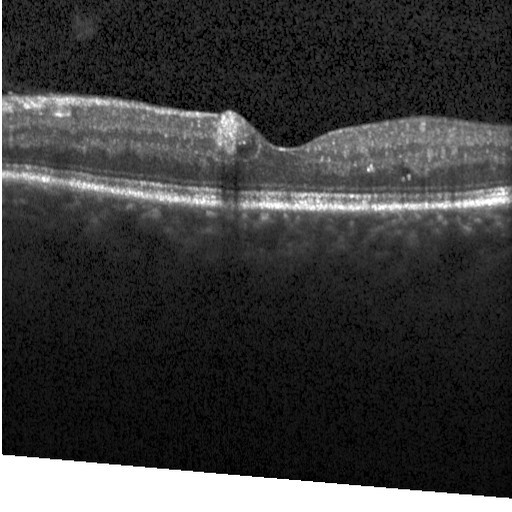

Heidelberg Spectralis, OCT B-scan. This B-scan demonstrates DME.